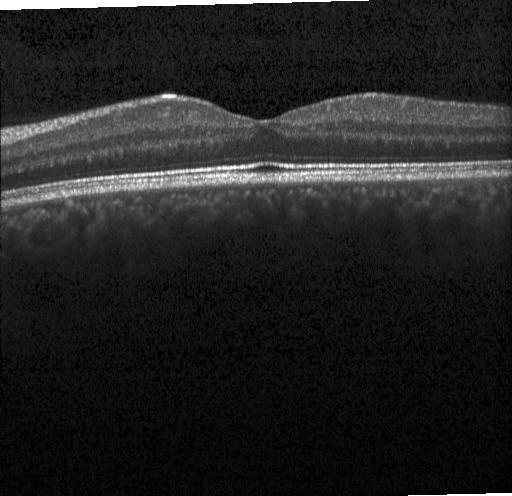

Optical coherence tomography scan, centered on the fovea, spectral-domain optical coherence tomography, acquired on a Heidelberg Spectralis.
Impression: no choroidal neovascularization, no diabetic macular edema, and no drusen.